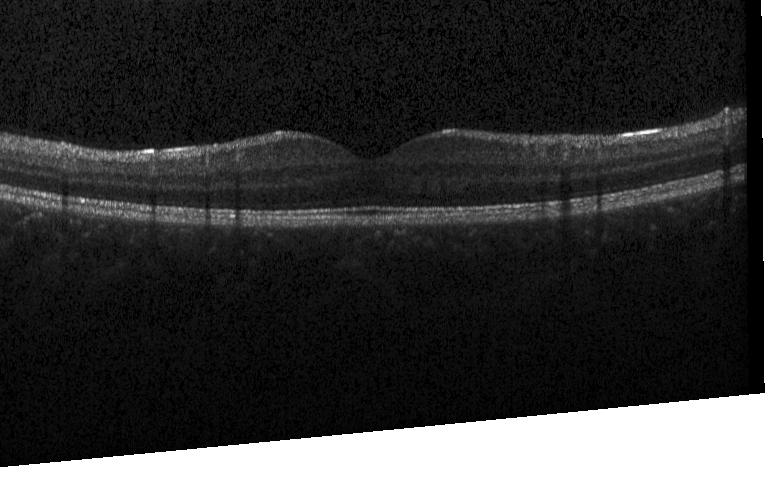
Diagnosis: no choroidal neovascularization, diabetic macular edema, or drusen.